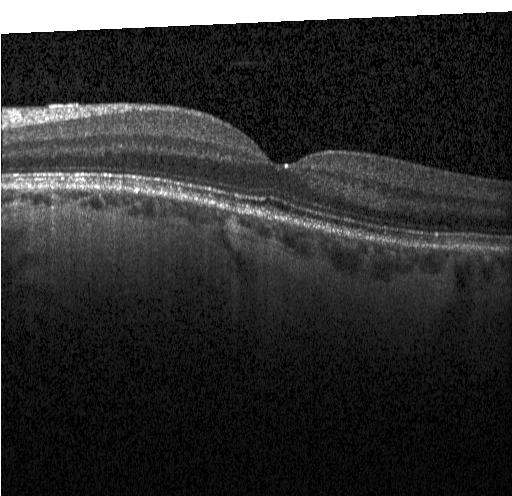
Spectral-domain OCT, retinal OCT B-scan. The scan shows no evidence of choroidal neovascularization, diabetic macular edema, or drusen.